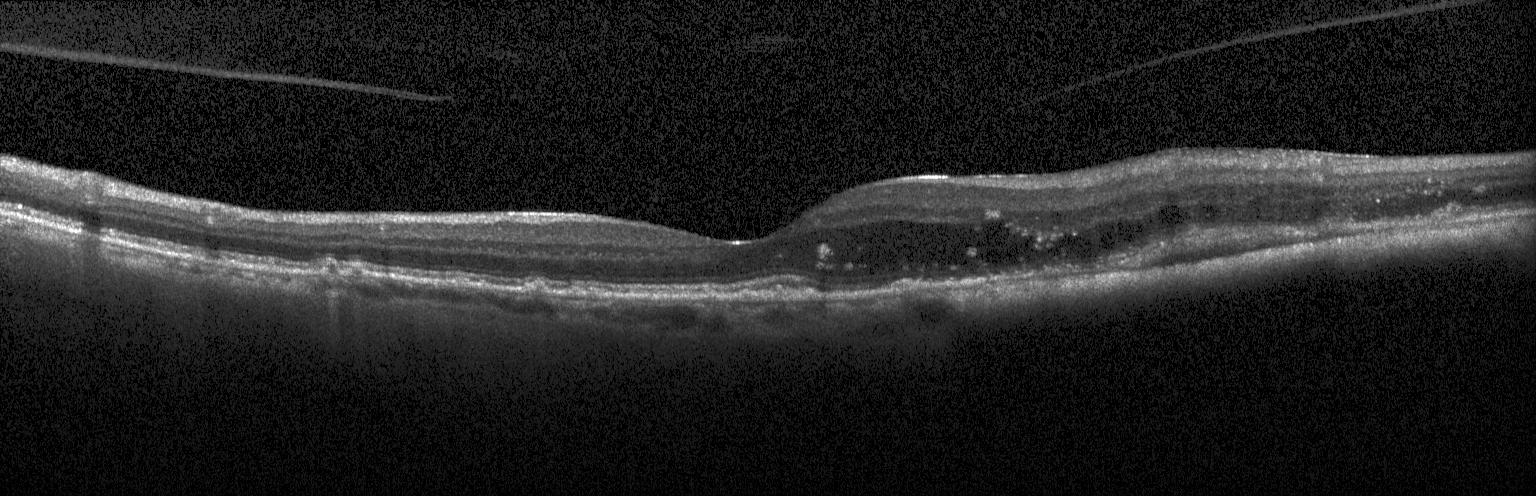 Retinal OCT B-scan; instrument: Heidelberg Spectralis; centered on the fovea; spectral-domain optical coherence tomography — Dx: a choroidal neovascular membrane.